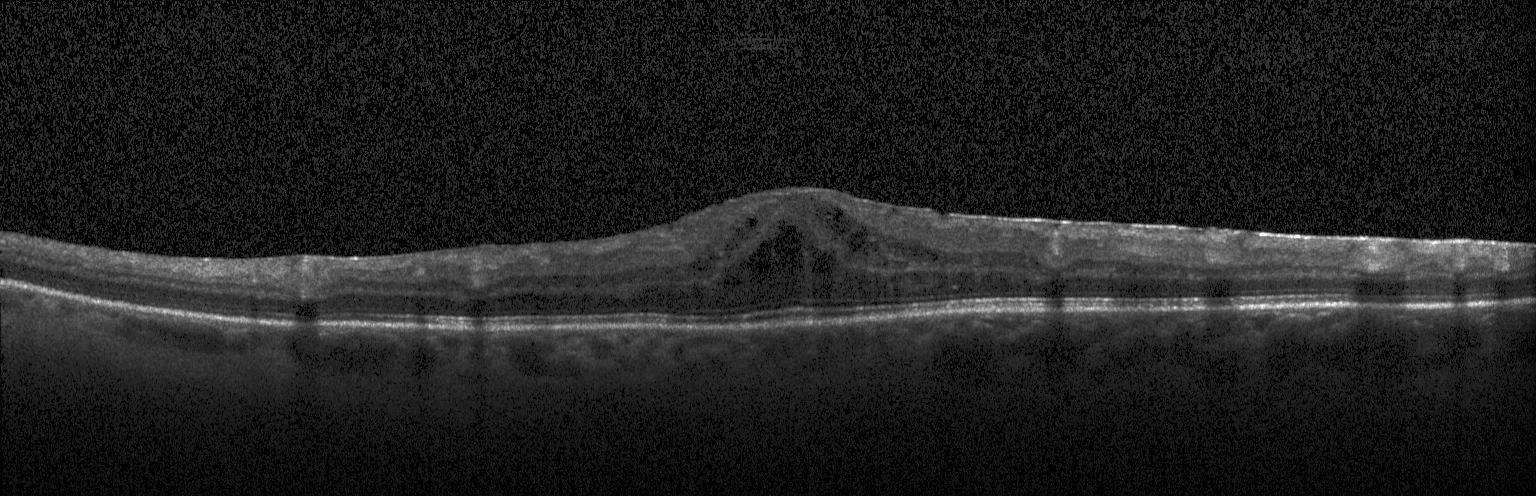
Diabetic macular edema.